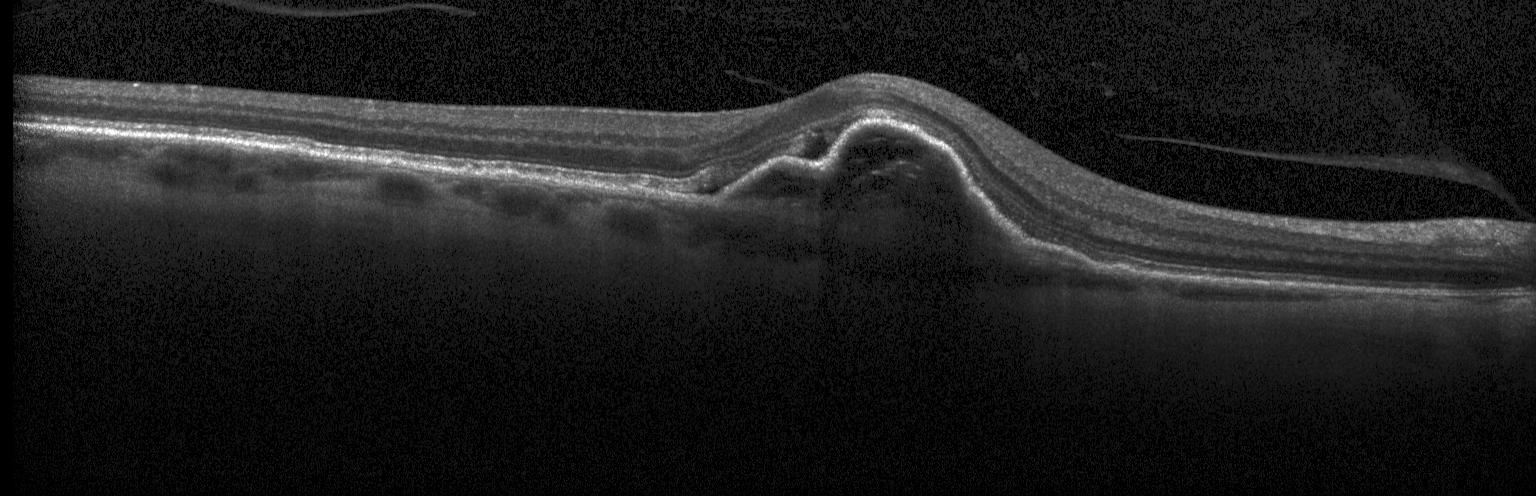 OCT line scan · spectral-domain OCT · through the macula · acquired on a Heidelberg Spectralis. Diagnosis: a choroidal neovascular membrane.